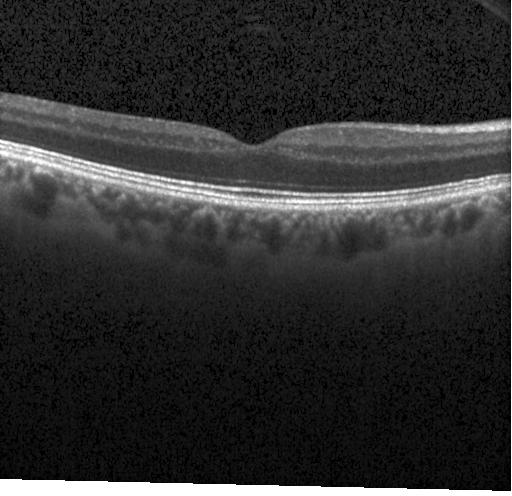

OCT finding: no choroidal neovascularization, no diabetic macular edema, and no drusen.